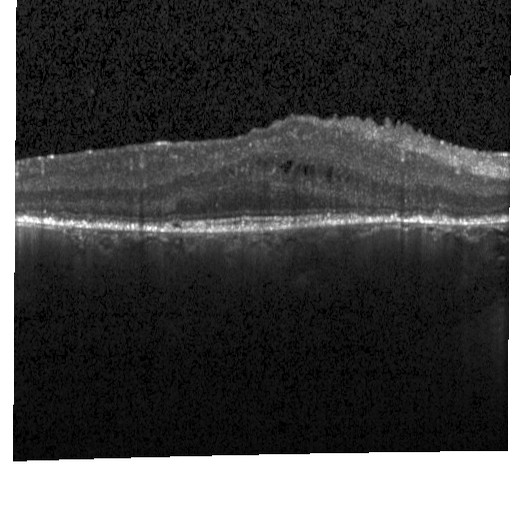 Macular scan · instrument: Heidelberg Spectralis · optical coherence tomography scan
The scan shows diabetic macular edema.